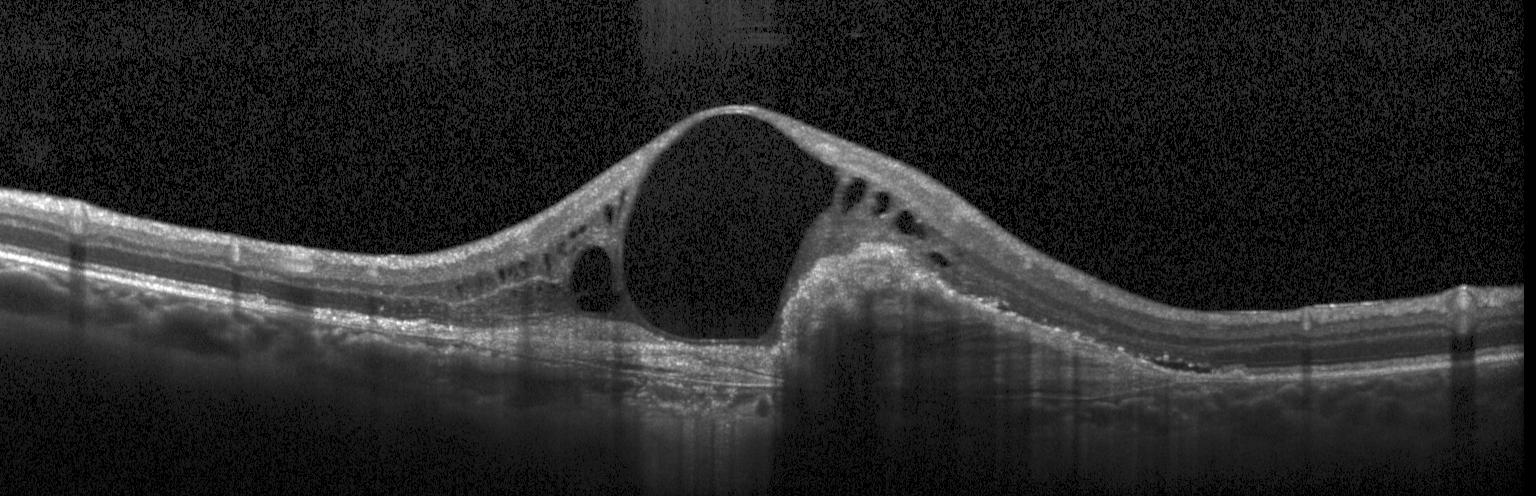 OCT B-scan showing CNV.